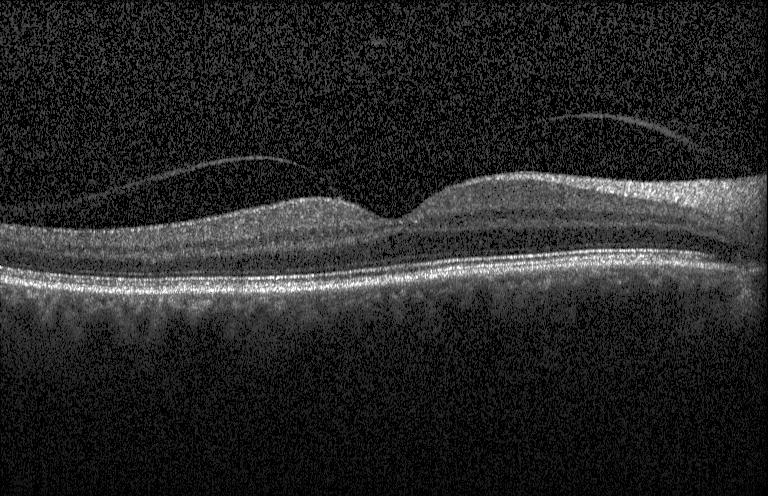

OCT B-scan. Through the macula. SD-OCT
Impression: no choroidal neovascularization, no diabetic macular edema, and no drusen.